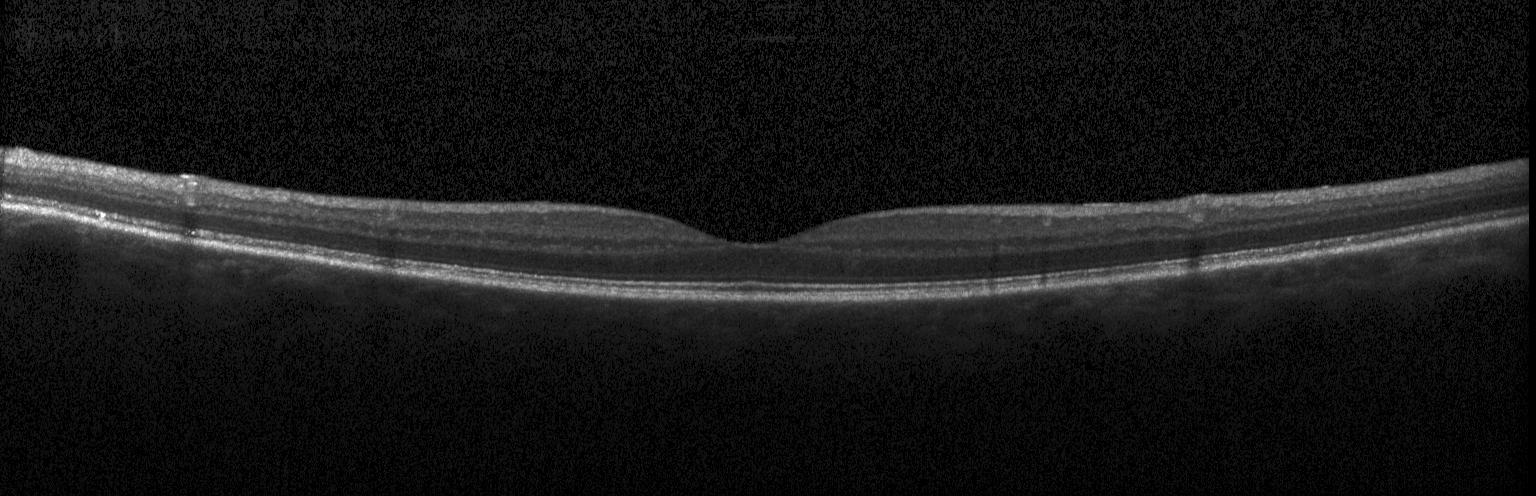
Fovea-centered. OCT line scan. Instrument: Heidelberg Spectralis. SD-OCT — This B-scan demonstrates no choroidal neovascularization, no diabetic macular edema, and no drusen.